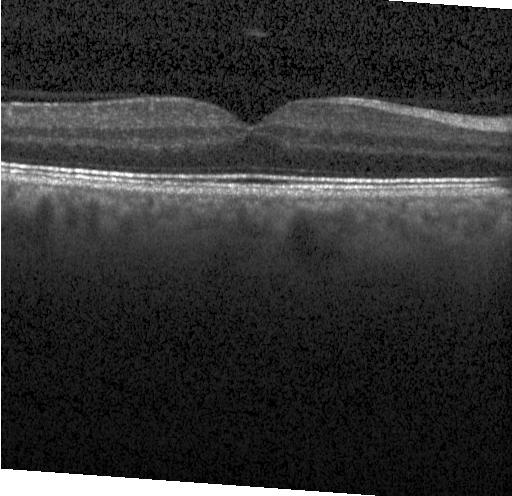 OCT B-scan.
Finding: no evidence of CNV, DME, or drusen.